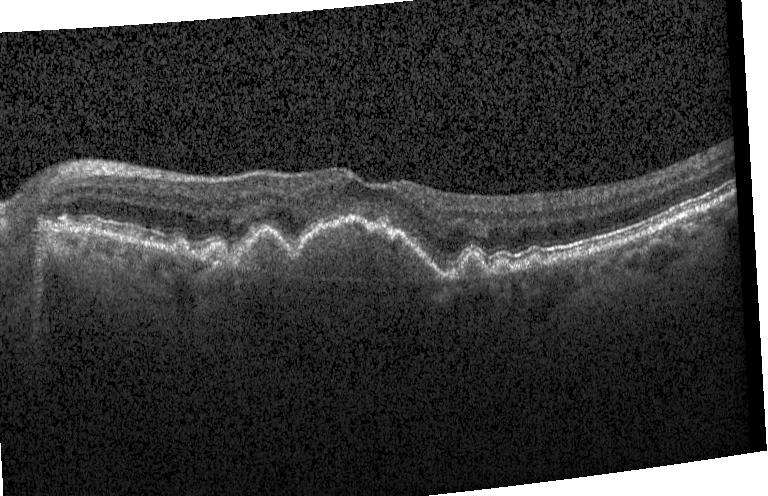

Dx: choroidal neovascularization.